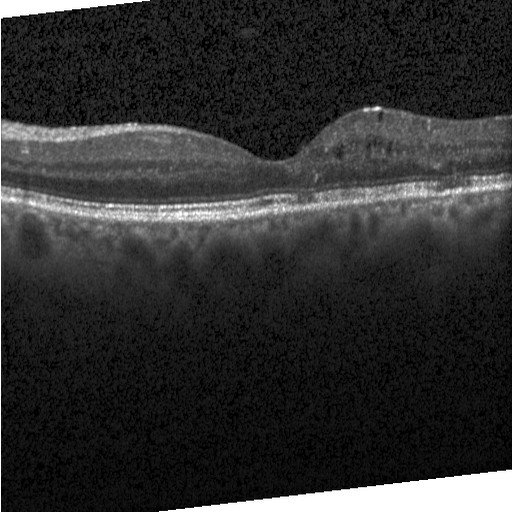 SD-OCT; OCT line scan; horizontal scan through the fovea.
Assessment: DME.